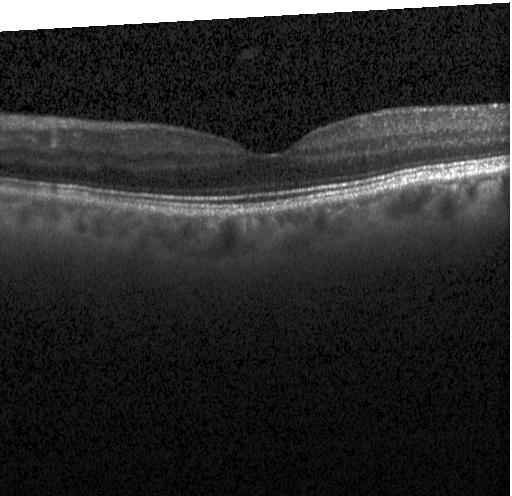
OCT line scan
Finding: no evidence of CNV, DME, or drusen.